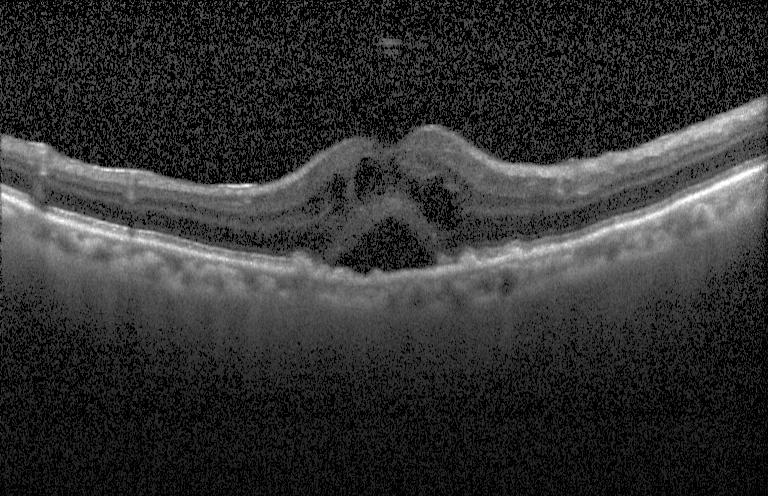
Retinal OCT cross-section. Diagnosis: diabetic macular edema.